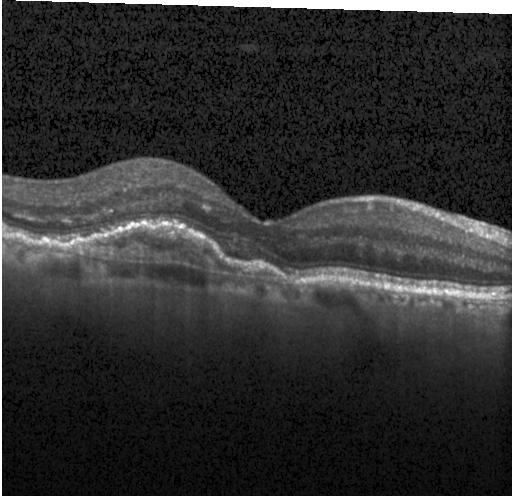
Macular OCT: choroidal neovascularization (CNV).